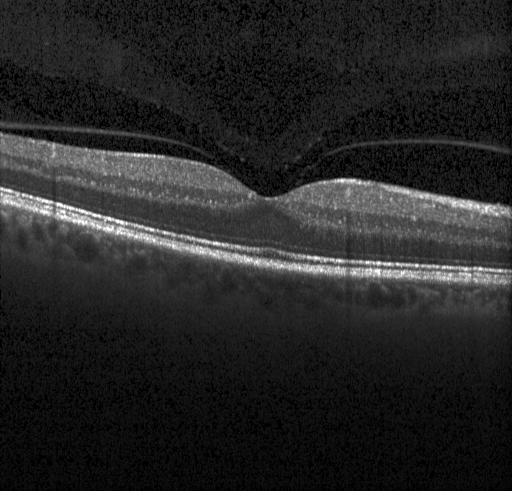
Assessment: no CNV, no DME, and no drusen.